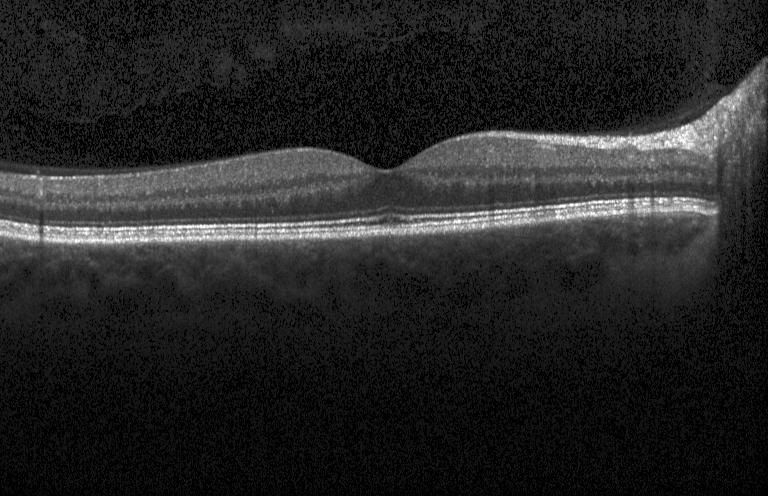
Finding: no CNV, no DME, and no drusen.